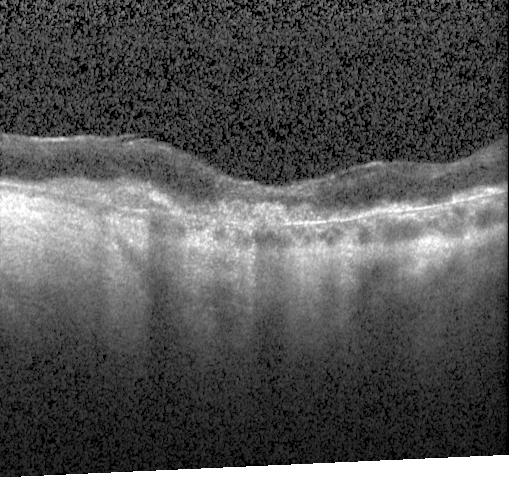

SD-OCT, OCT B-scan, through the macula, acquired on a Heidelberg Spectralis. Impression: choroidal neovascularization.